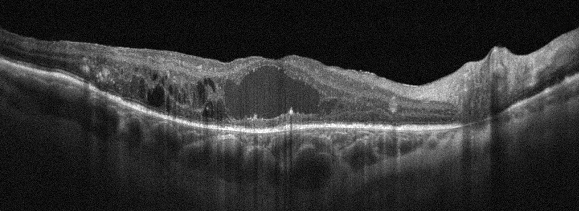

Through the macula. Acquired on an Optovue Avanti RTVue XR. OCT line scan
The scan shows diabetic macular edema.